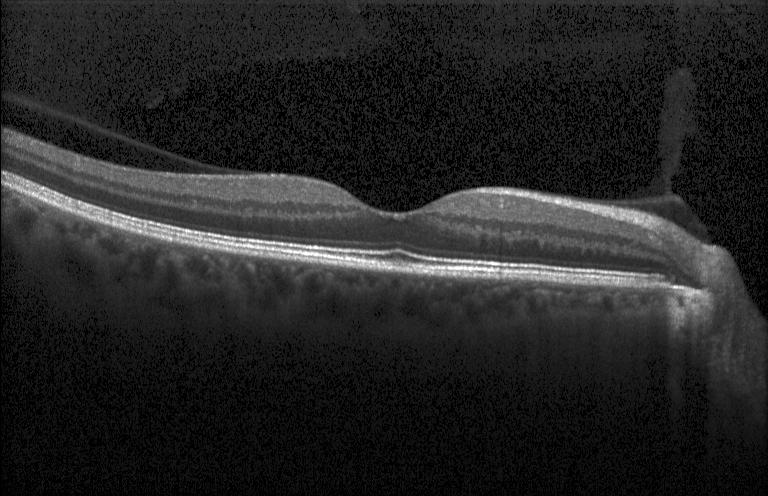

Macular OCT demonstrating no choroidal neovascularization, no diabetic macular edema, and no drusen.